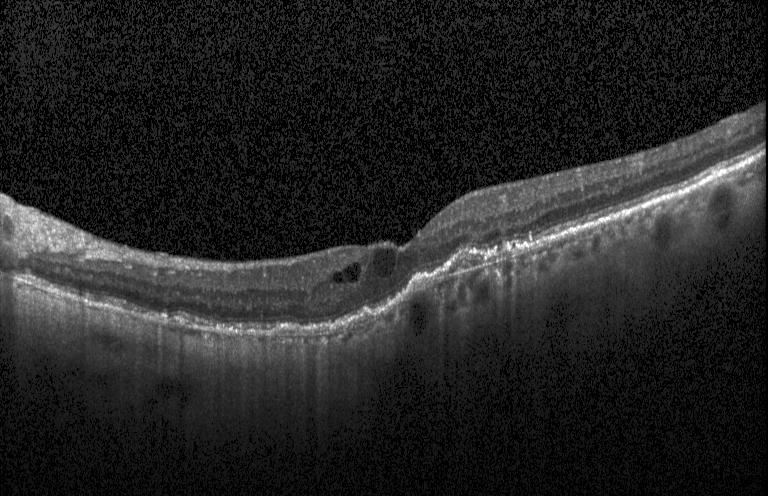
Instrument: Heidelberg Spectralis. Optical coherence tomography B-scan
The scan shows a choroidal neovascular membrane.